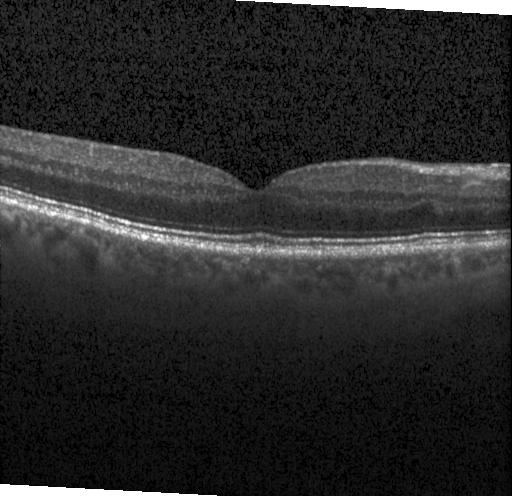

Retinal OCT cross-section · Heidelberg Spectralis — This B-scan demonstrates no CNV, no DME, and no drusen.